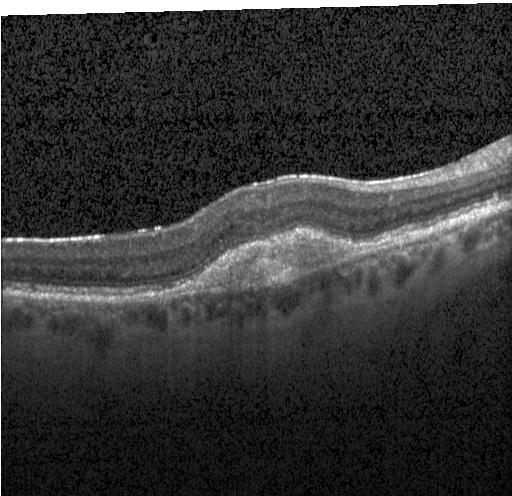
OCT B-scan showing a choroidal neovascular membrane.